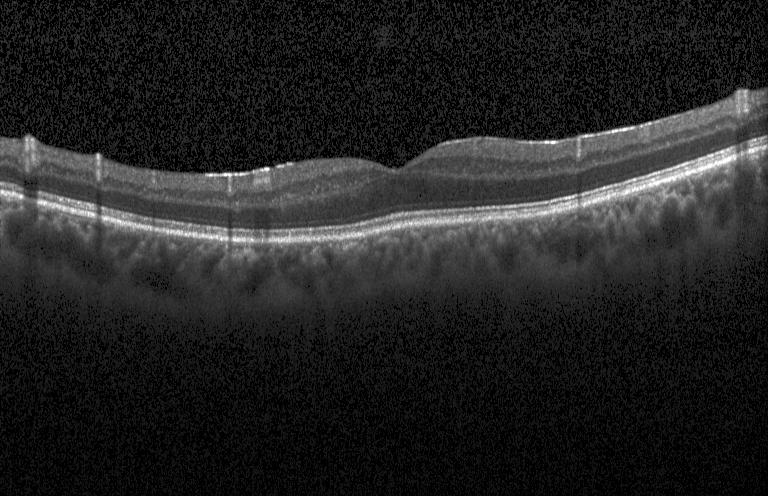 The scan shows no evidence of CNV, DME, or drusen.